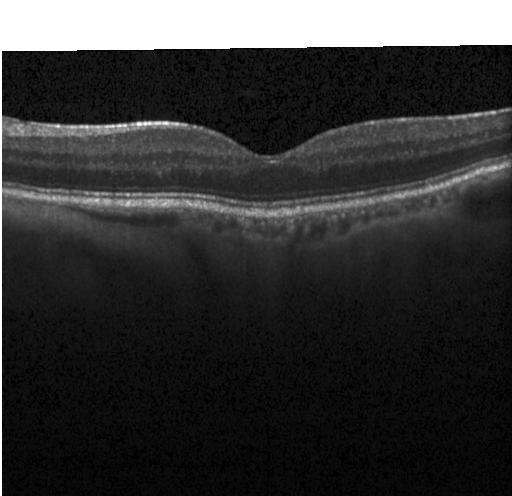
OCT B-scan · spectral-domain optical coherence tomography.
Finding: neither CNV, DME, nor drusen.